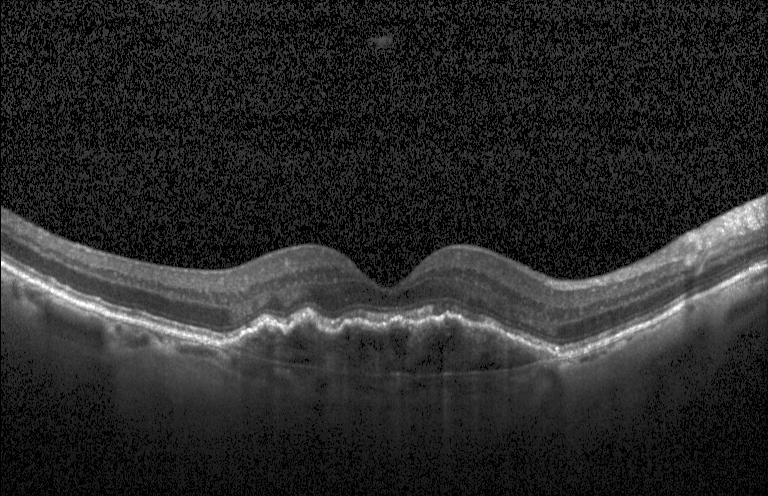 OCT B-scan · Heidelberg Spectralis.
Finding: choroidal neovascularization (CNV).